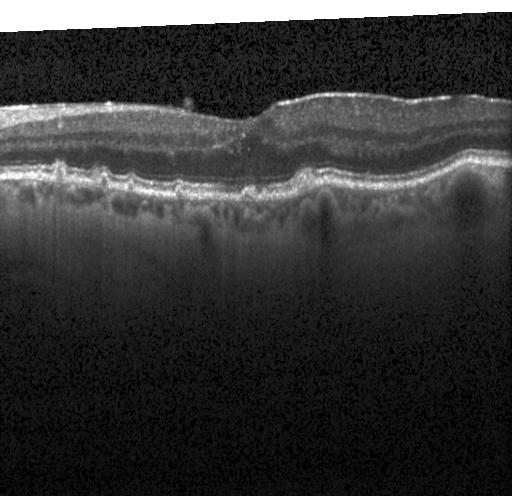 Retinal OCT B-scan. The scan shows drusen.